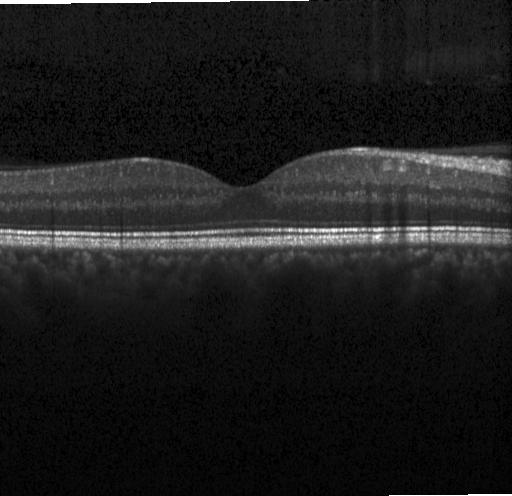

Impression: no CNV, DME, or drusen.